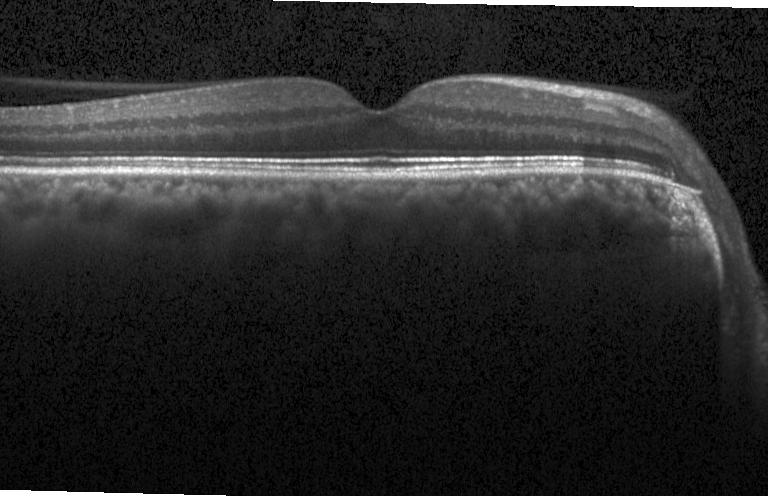 Assessment: no evidence of CNV, DME, or drusen.